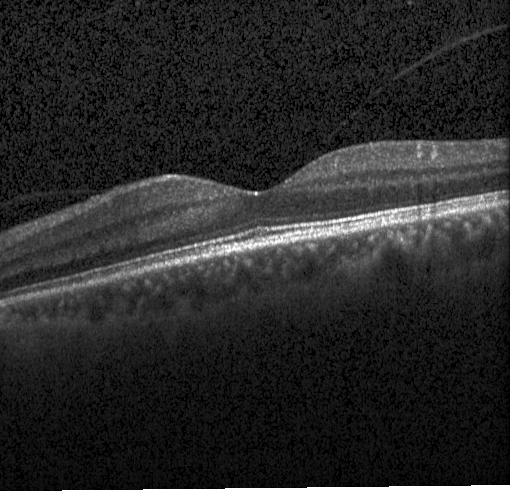 Macular OCT demonstrating no CNV, no DME, and no drusen.